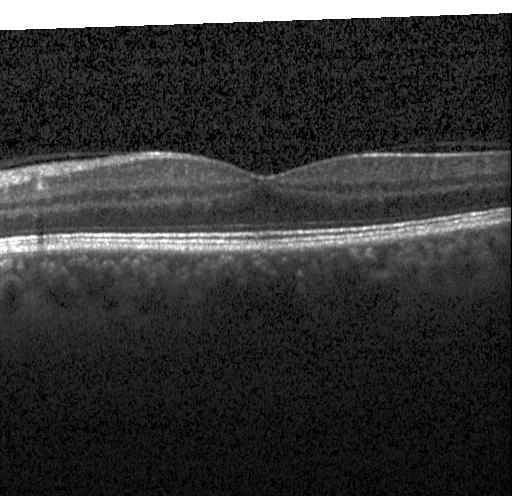 Optical coherence tomography B-scan.
This B-scan demonstrates no choroidal neovascularization, diabetic macular edema, or drusen.